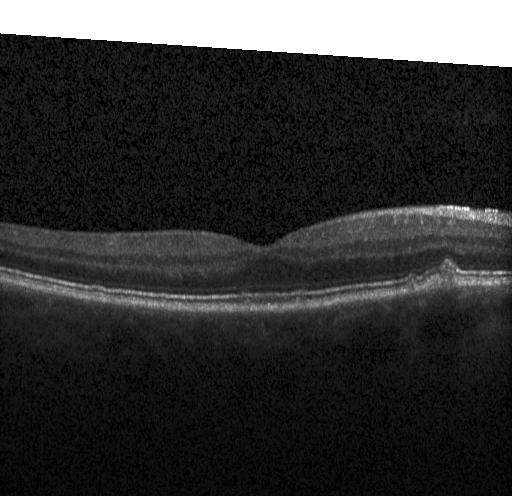
Spectral-domain optical coherence tomography · optical coherence tomography scan. Impression: multiple drusen.